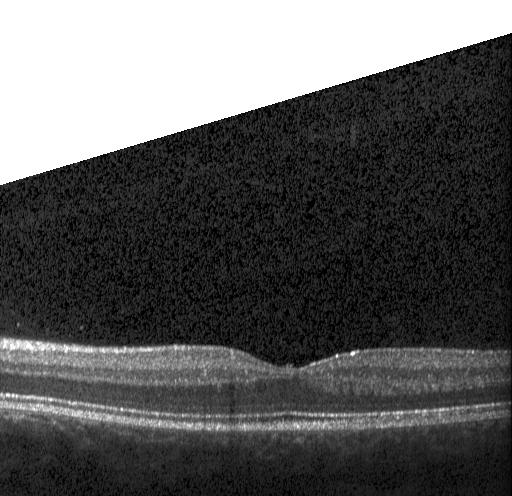

OCT B-scan. Instrument: Heidelberg Spectralis. Diagnosis: no evidence of CNV, DME, or drusen.